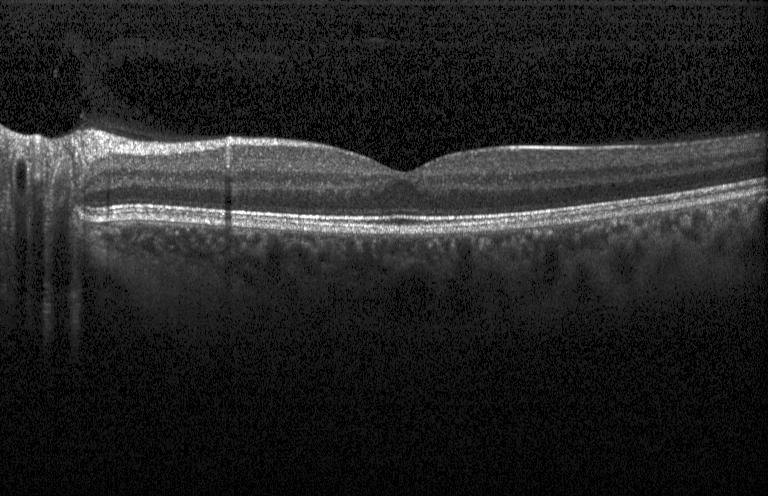 This B-scan demonstrates no CNV, no DME, and no drusen.